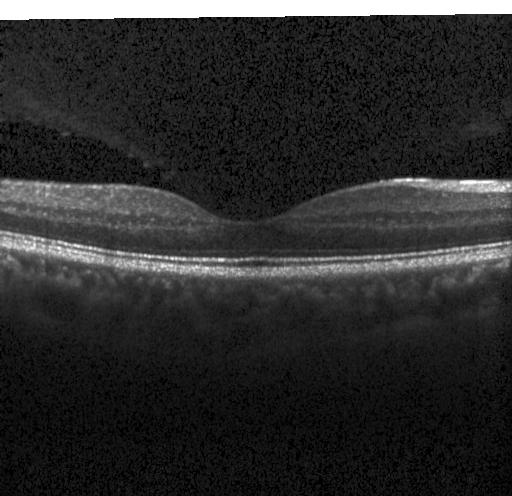

Optical coherence tomography B-scan · Heidelberg Spectralis. This B-scan demonstrates no evidence of choroidal neovascularization, diabetic macular edema, or drusen.